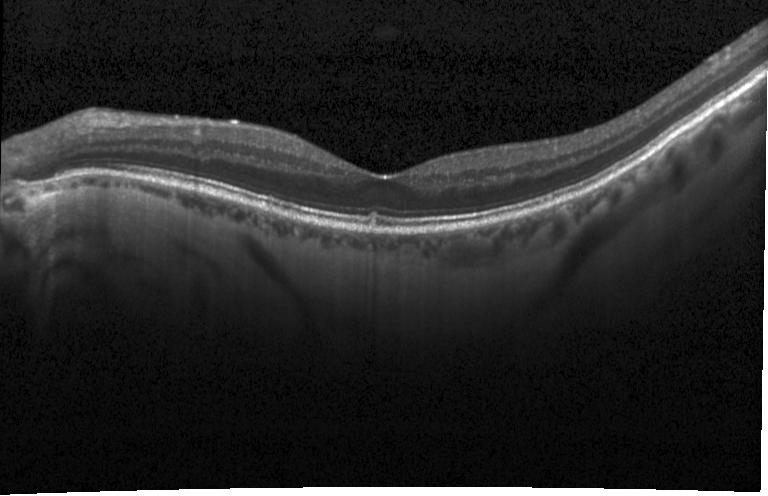
Spectral-domain OCT. Retinal OCT B-scan. Acquired on a Heidelberg Spectralis. Through the macula
Assessment: sub-RPE drusenoid deposits.